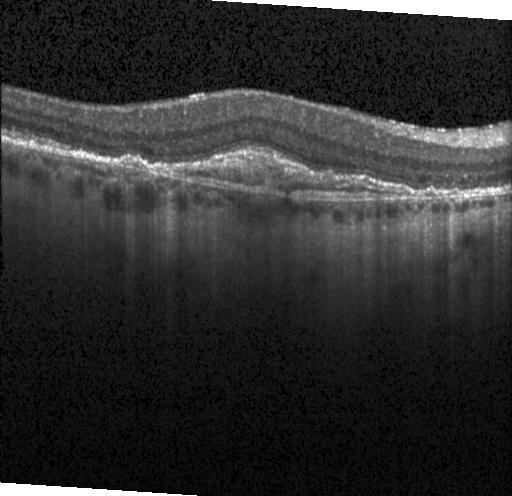

Macular OCT demonstrating a choroidal neovascular membrane.